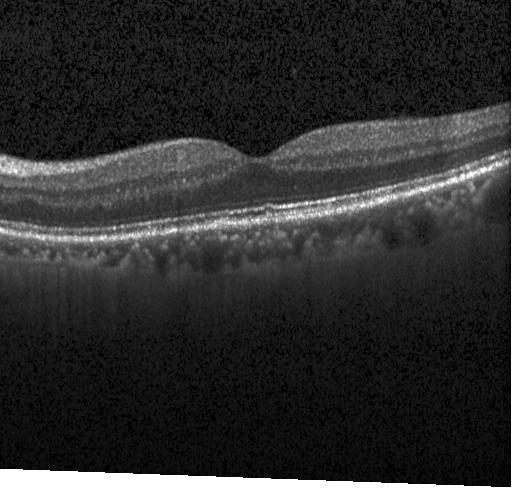
OCT B-scan
The scan shows no choroidal neovascularization, no diabetic macular edema, and no drusen.